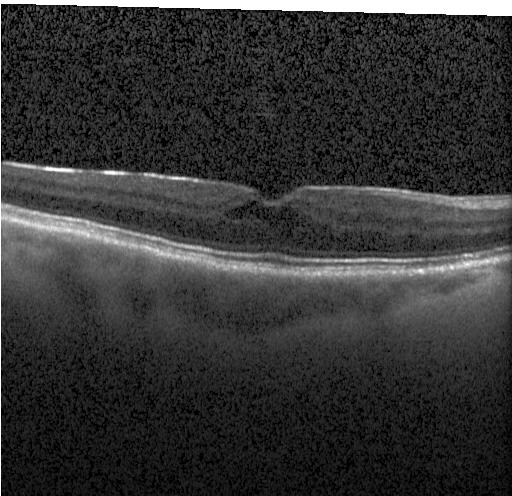 OCT finding: DME.